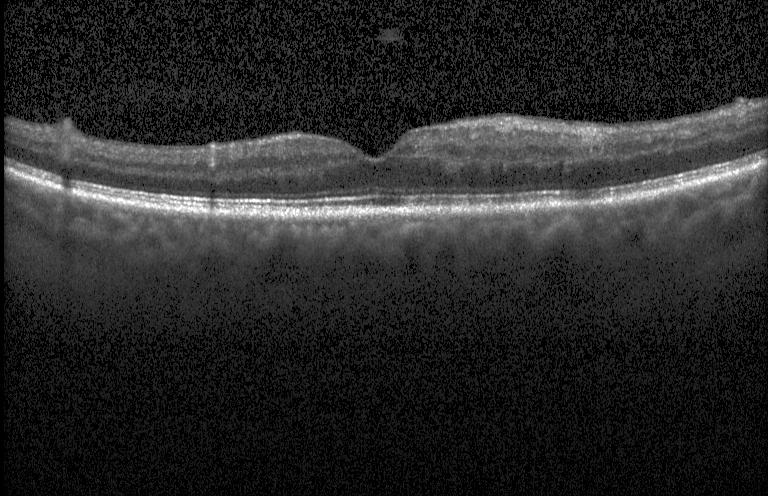
The scan shows neither choroidal neovascularization, diabetic macular edema, nor drusen.